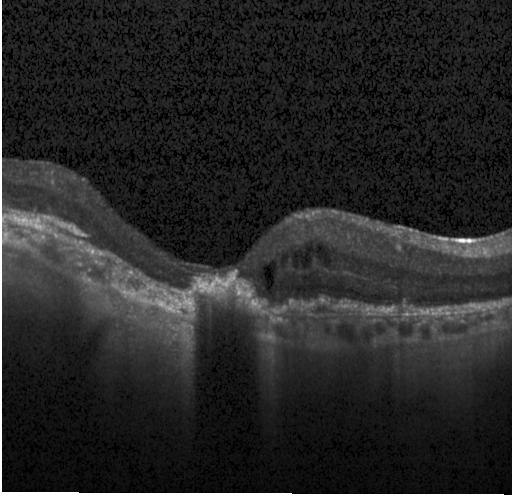
Diagnosis: CNV.